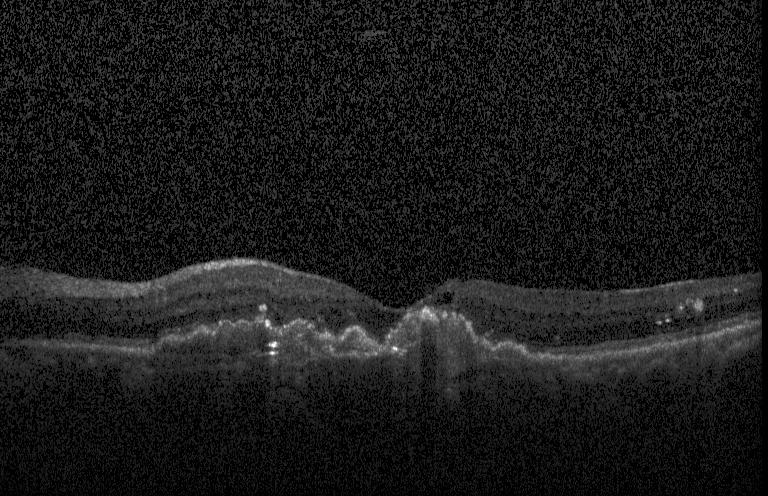

Optical coherence tomography scan. Macular scan
A choroidal neovascular membrane.